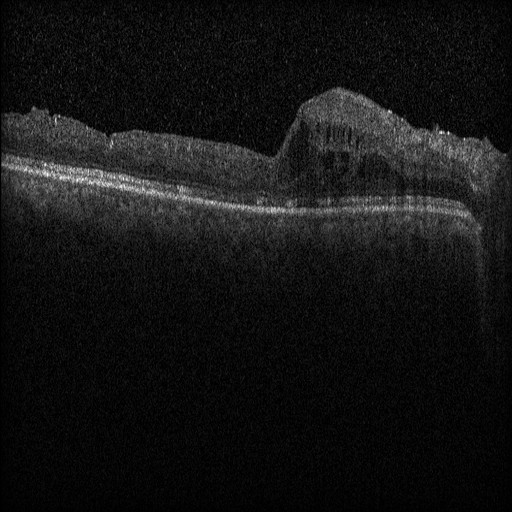 Retinal OCT cross-section showing diabetic macular edema.